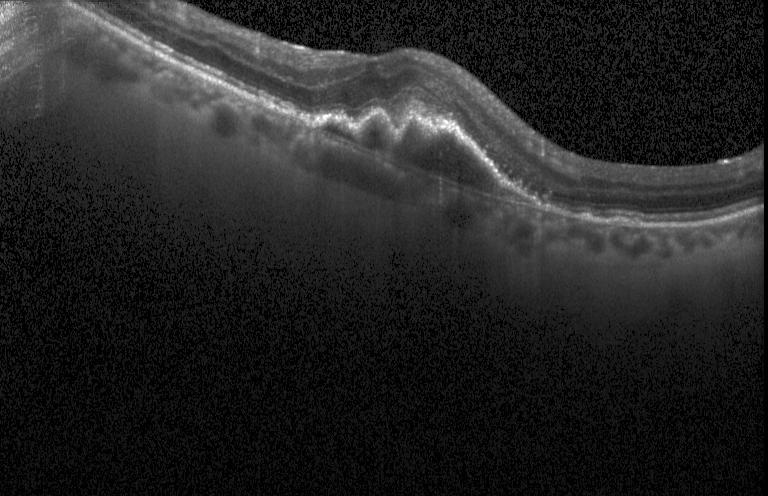 Spectral-domain OCT · optical coherence tomography scan — The scan shows a choroidal neovascular membrane.